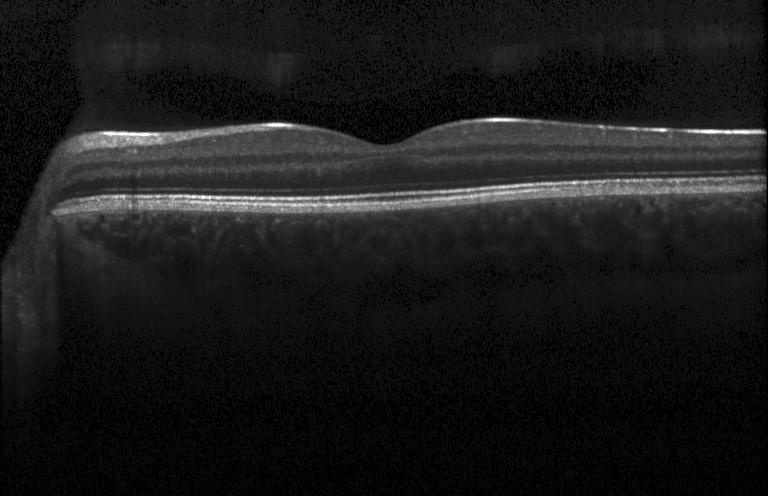 Impression: no evidence of choroidal neovascularization, diabetic macular edema, or drusen.